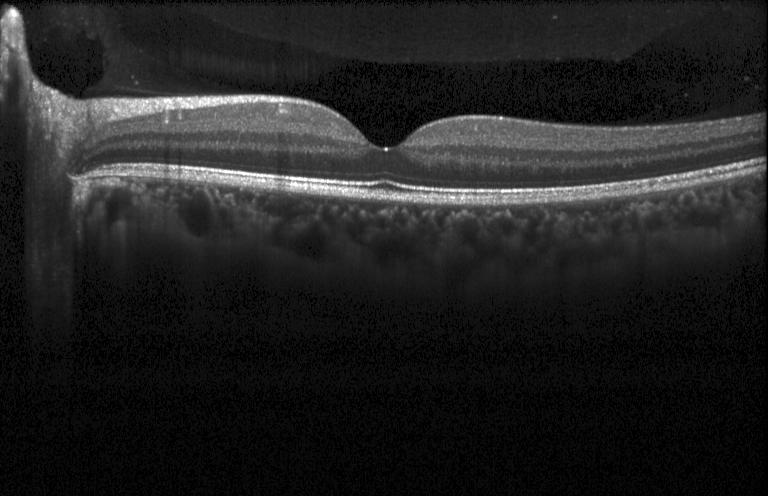

OCT B-scan
Macular OCT: neither CNV, DME, nor drusen.